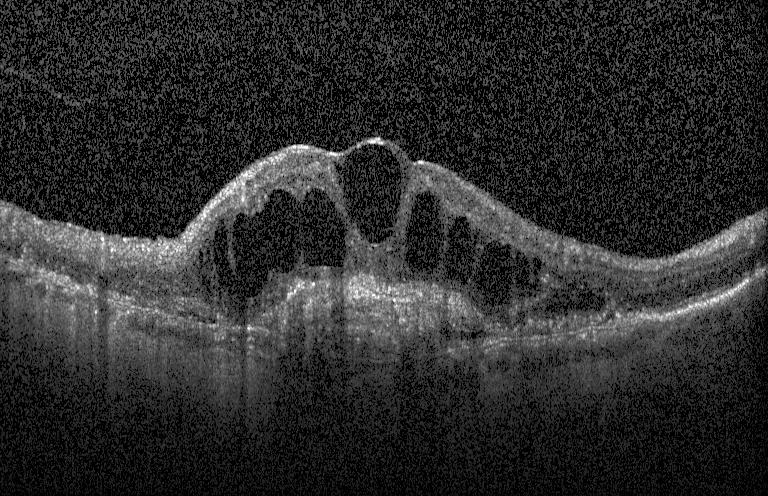
Diagnosis: a choroidal neovascular membrane.